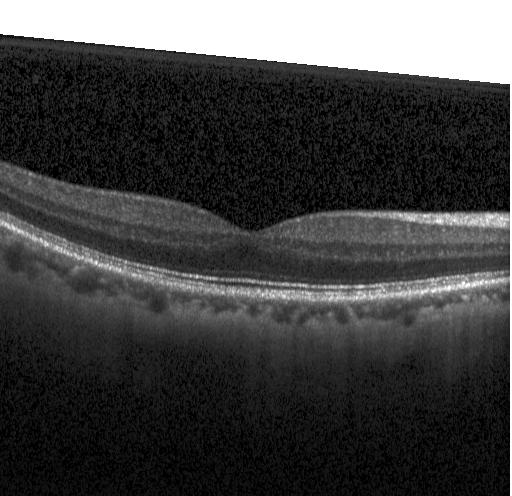 OCT finding: no CNV, no DME, and no drusen.